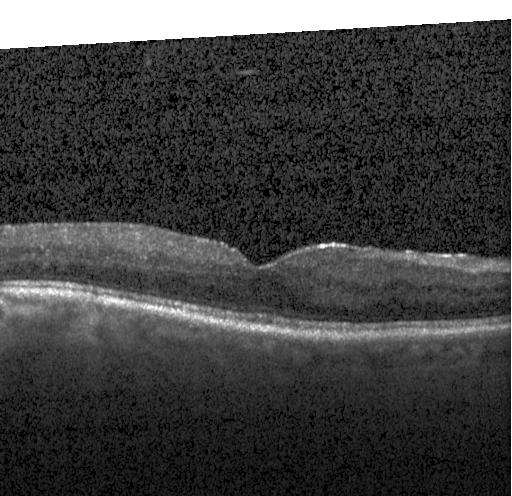 Retinal OCT cross-section
Finding: no evidence of CNV, DME, or drusen.